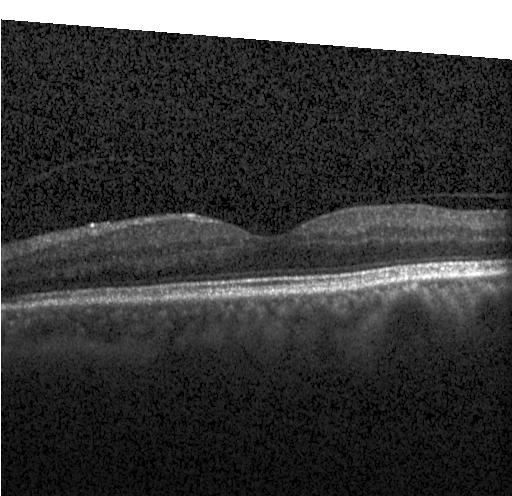 Assessment: no choroidal neovascularization, no diabetic macular edema, and no drusen.